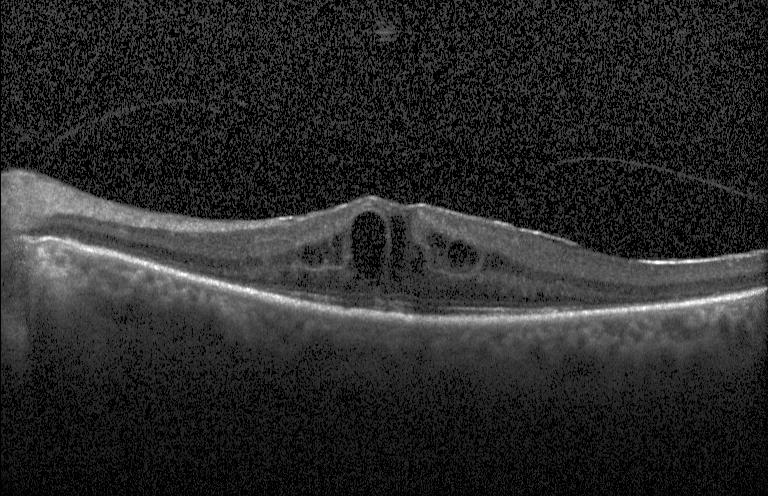

Optical coherence tomography B-scan. Spectral-domain optical coherence tomography. Fovea-centered. Instrument: Heidelberg Spectralis
The scan shows diabetic macular edema (DME).